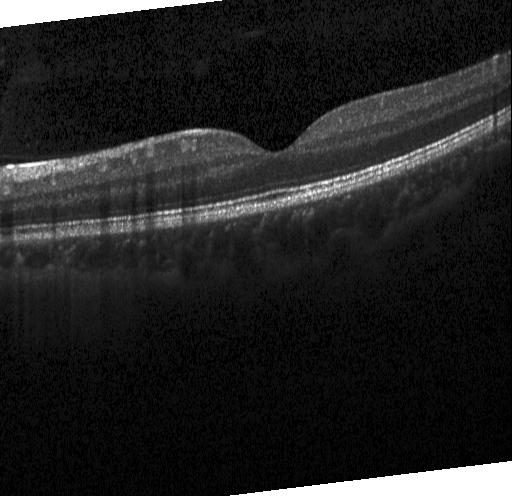
OCT line scan. Instrument: Heidelberg Spectralis. Spectral-domain OCT — Diagnosis: no choroidal neovascularization, diabetic macular edema, or drusen.